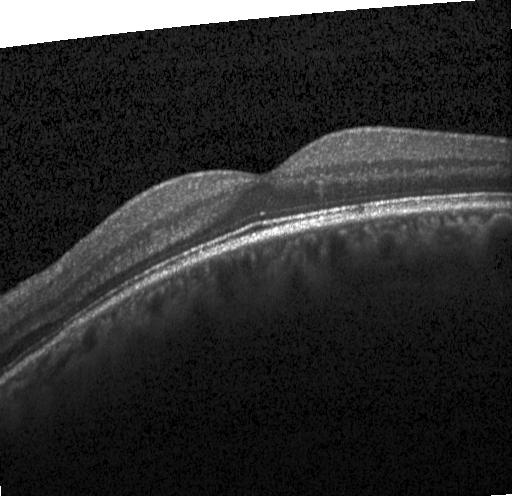 Heidelberg Spectralis OCT system, macular scan, retinal OCT B-scan, spectral-domain optical coherence tomography
The scan shows no choroidal neovascularization, diabetic macular edema, or drusen.